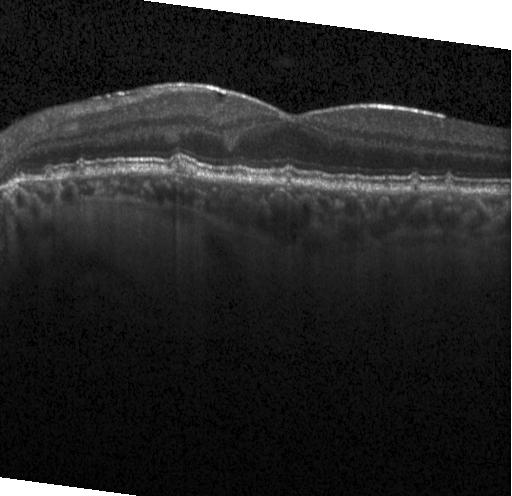 Spectral-domain OCT, retinal OCT cross-section, Heidelberg Spectralis, fovea-centered. Finding: sub-RPE drusenoid deposits.